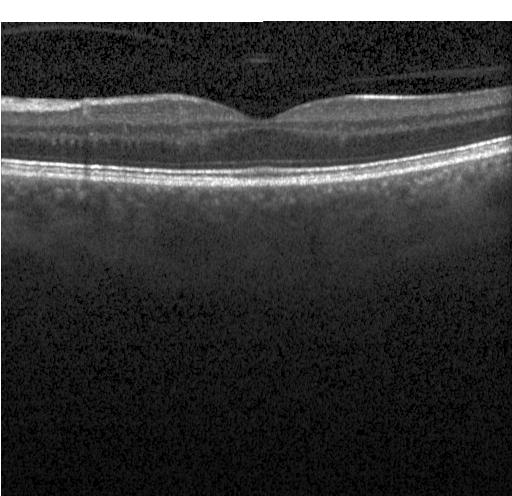
OCT B-scan; Heidelberg Spectralis OCT system; macular scan.
No CNV, no DME, and no drusen.